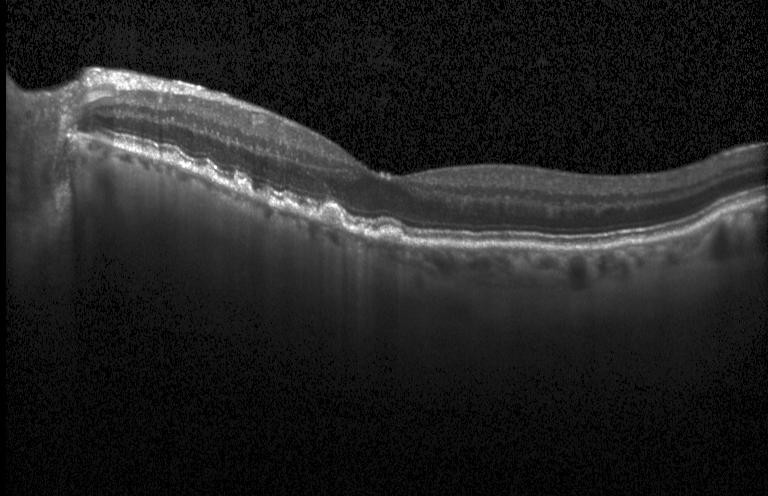
OCT finding: multiple drusen.